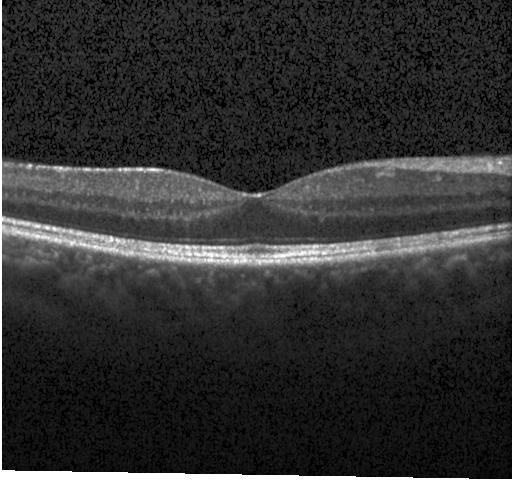 Assessment: no choroidal neovascularization, no diabetic macular edema, and no drusen.